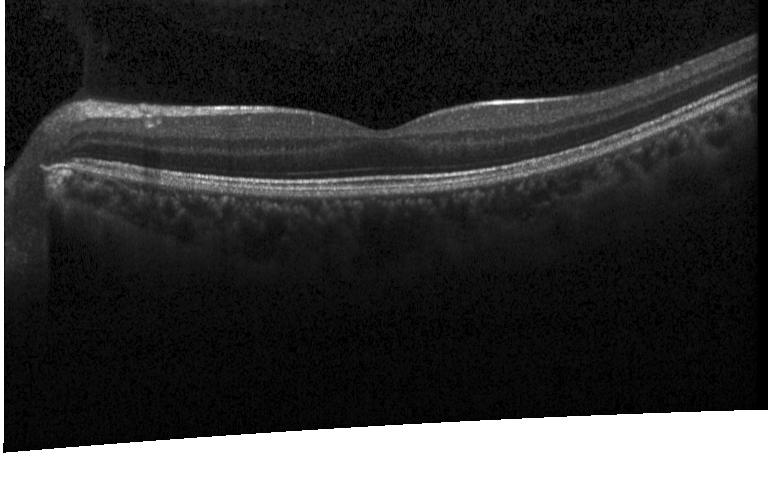 Spectral-domain optical coherence tomography, Heidelberg Spectralis OCT system, optical coherence tomography scan, macular scan. This B-scan demonstrates no choroidal neovascularization, diabetic macular edema, or drusen.